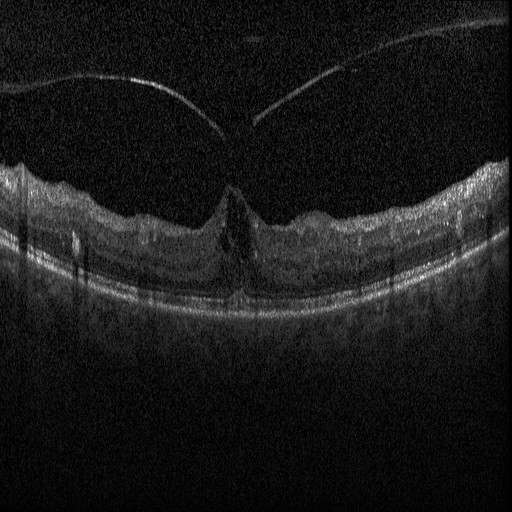
OCT B-scan. Fovea-centered — Diagnosis: diabetic macular edema.